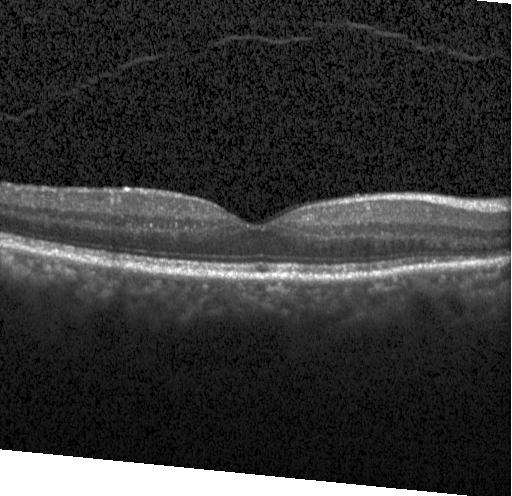 Optical coherence tomography B-scan — No choroidal neovascularization, no diabetic macular edema, and no drusen.